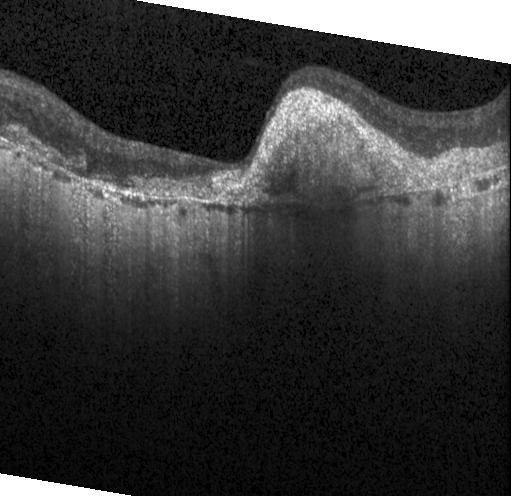 Instrument: Heidelberg Spectralis. Optical coherence tomography scan. OCT finding: a choroidal neovascular membrane.